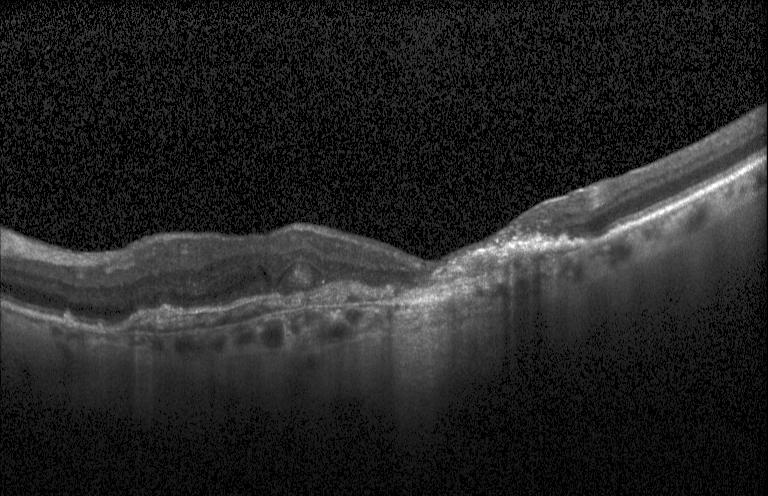

Impression: a choroidal neovascular membrane.